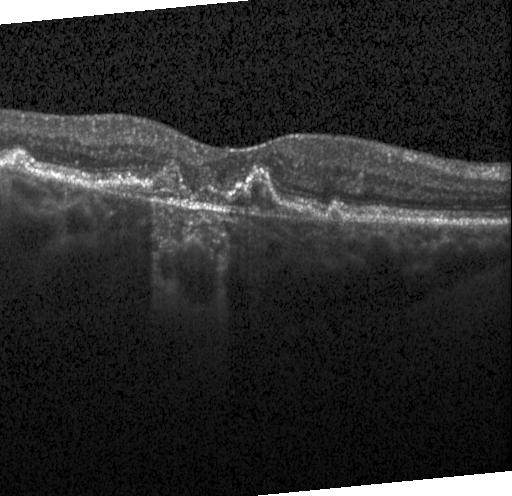
Spectral-domain OCT; retinal OCT cross-section.
Dx: choroidal neovascularization (CNV).